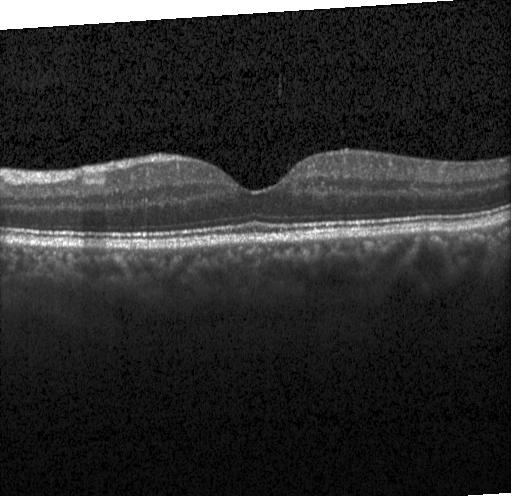
Through the macula, retinal OCT B-scan, spectral-domain optical coherence tomography — Finding: neither choroidal neovascularization, diabetic macular edema, nor drusen.